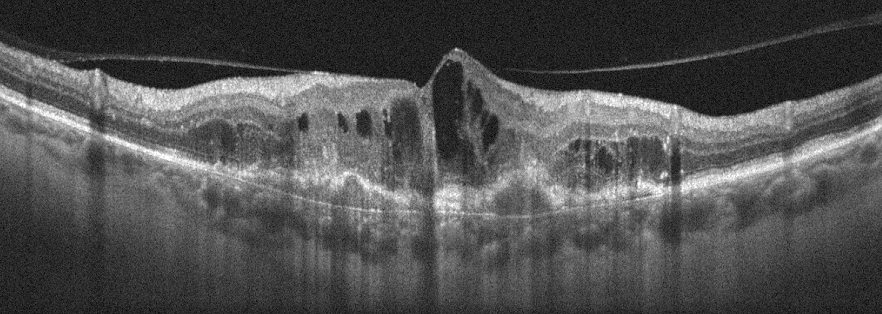
Optical coherence tomography B-scan · left eye — The scan shows age-related macular degeneration (AMD).